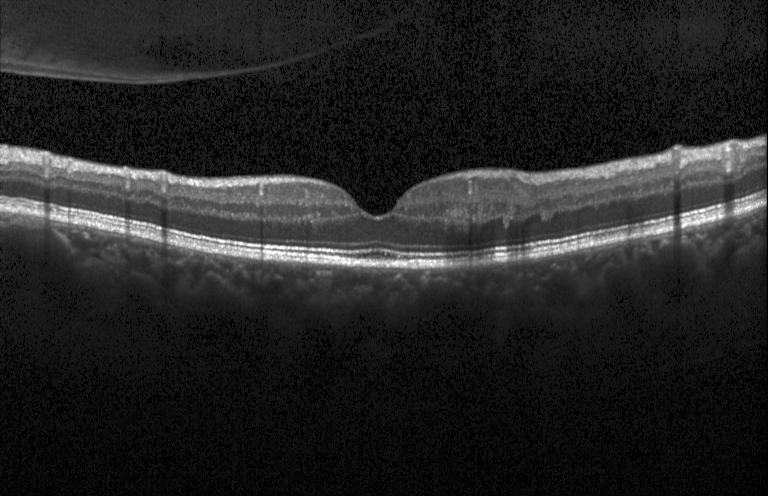 Heidelberg Spectralis OCT system · spectral-domain optical coherence tomography · optical coherence tomography B-scan.
Macular OCT: no choroidal neovascularization, no diabetic macular edema, and no drusen.